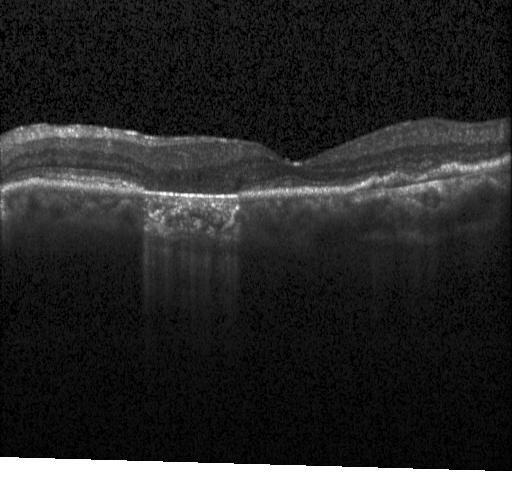

Assessment: a choroidal neovascular membrane.